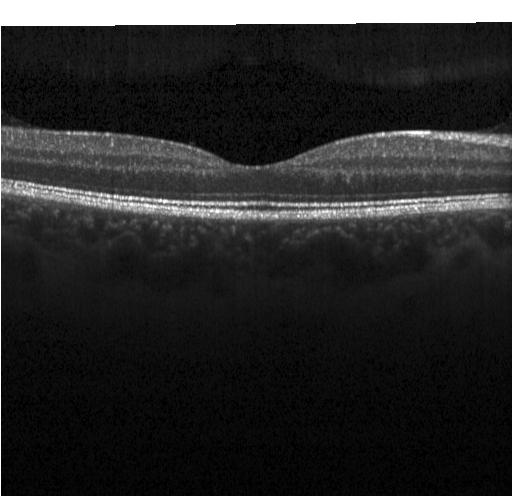
Through the macula; retinal OCT B-scan; spectral-domain OCT; instrument: Heidelberg Spectralis
Diagnosis: no choroidal neovascularization, diabetic macular edema, or drusen.